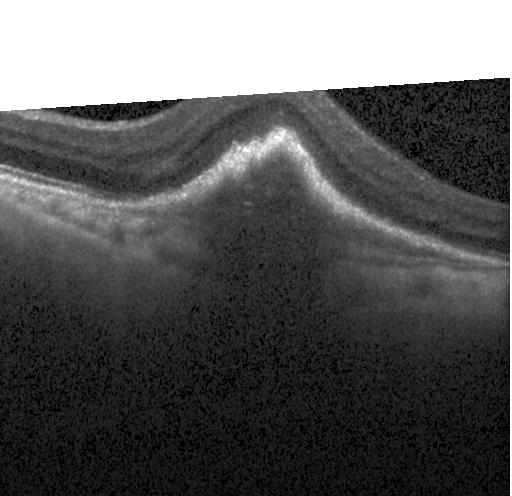 OCT B-scan showing a choroidal neovascular membrane.